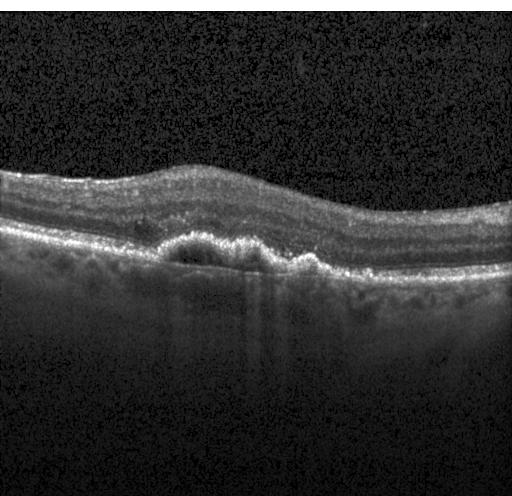 Optical coherence tomography B-scan. Spectral-domain optical coherence tomography. Fovea-centered. Heidelberg Spectralis OCT system. Dx: a choroidal neovascular membrane.